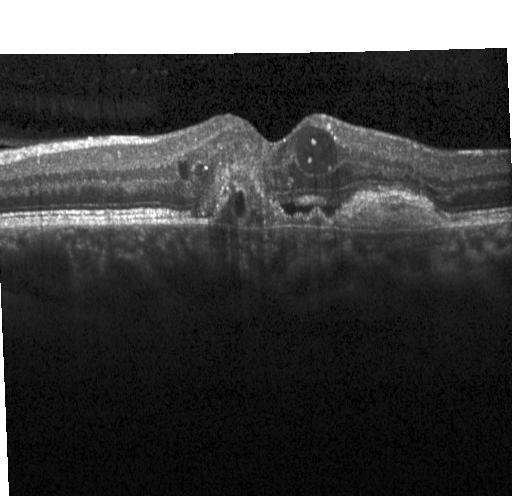
OCT line scan. Centered on the fovea. This B-scan demonstrates a choroidal neovascular membrane.